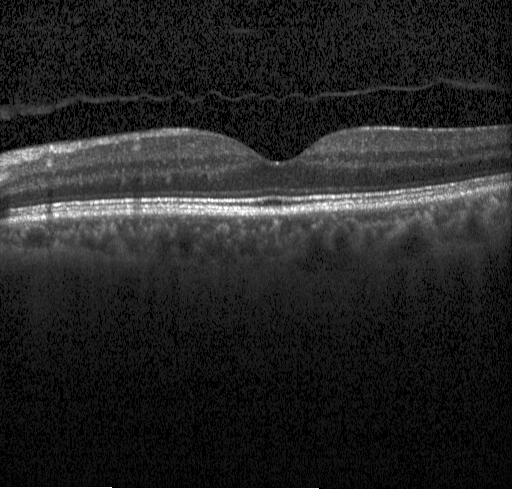 Impression: no choroidal neovascularization, diabetic macular edema, or drusen.